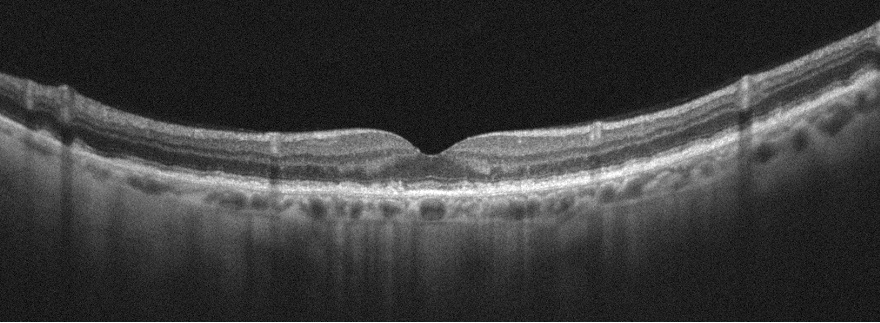
Macular OCT: AMD.